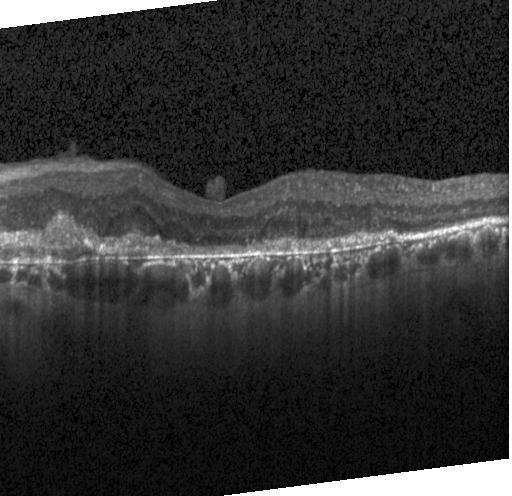

Acquired on a Heidelberg Spectralis. OCT line scan. Spectral-domain optical coherence tomography. Fovea-centered.
This B-scan demonstrates a choroidal neovascular membrane.